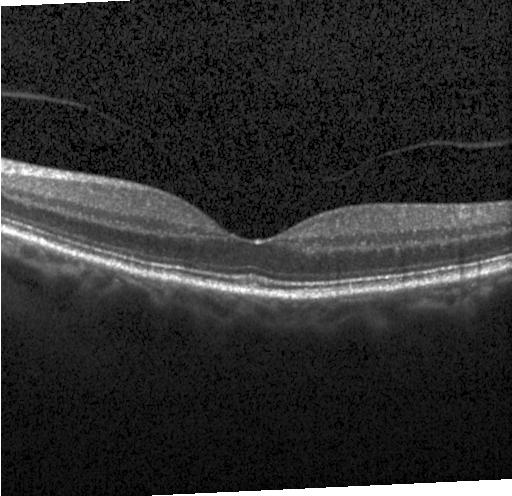

Retinal OCT B-scan — This B-scan demonstrates neither CNV, DME, nor drusen.